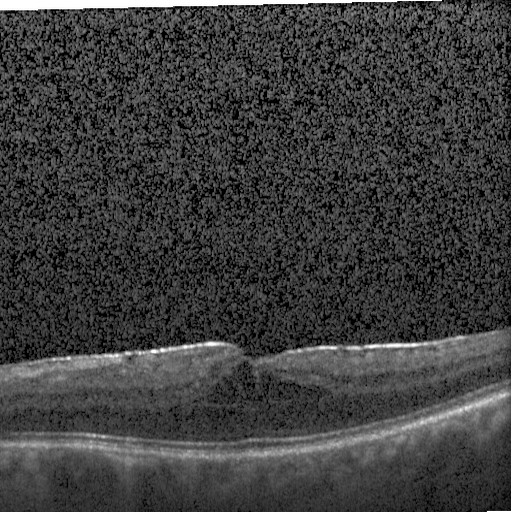

OCT scan showing diabetic macular edema (DME).